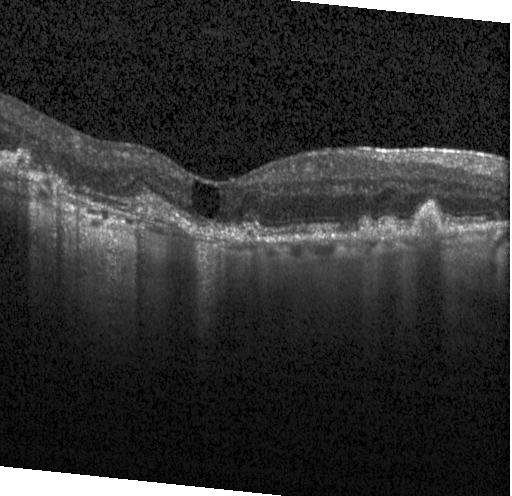 OCT B-scan showing CNV.